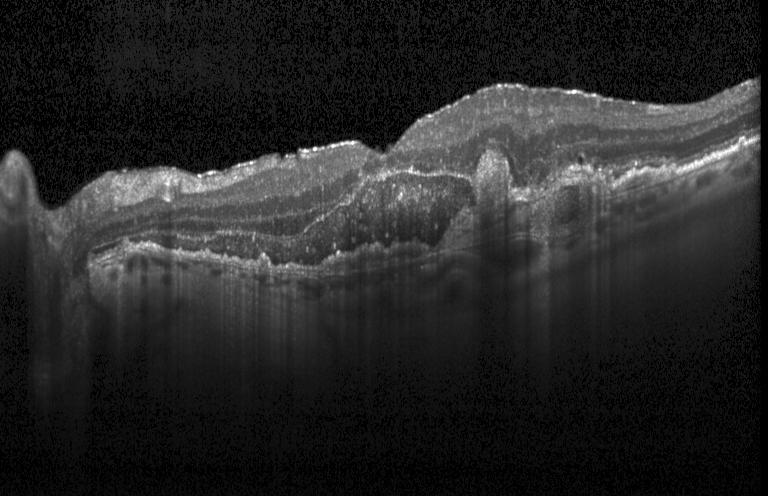 SD-OCT; macular scan; Heidelberg Spectralis OCT system; retinal OCT cross-section. Impression: a choroidal neovascular membrane.